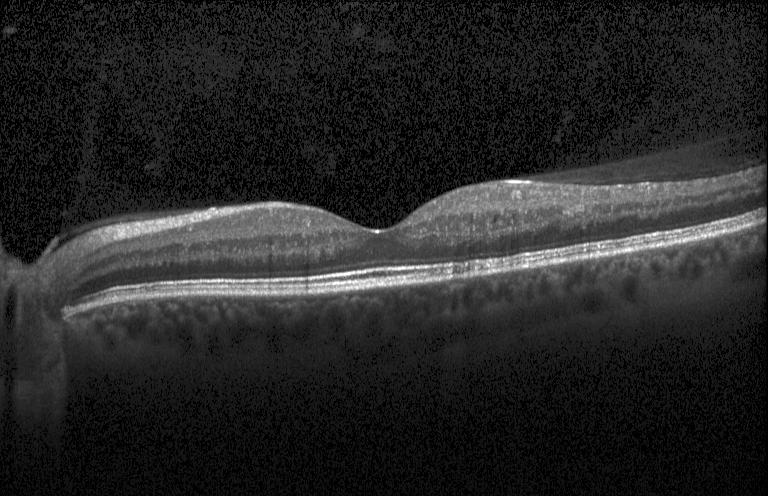 This B-scan demonstrates no evidence of CNV, DME, or drusen.